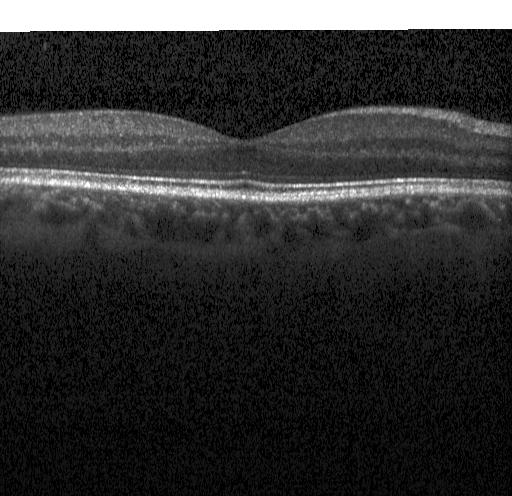

SD-OCT. Instrument: Heidelberg Spectralis. Fovea-centered. Optical coherence tomography scan — Impression: no choroidal neovascularization, diabetic macular edema, or drusen.